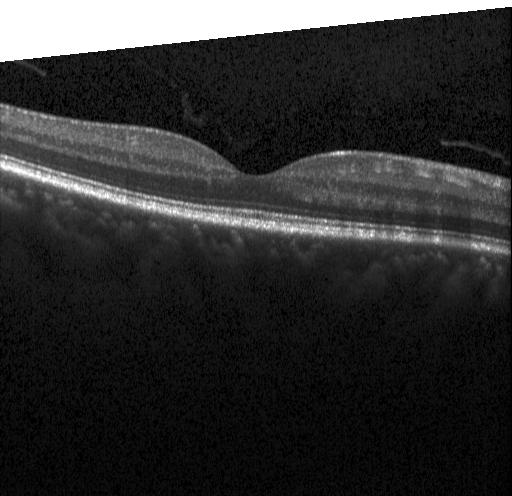 SD-OCT; optical coherence tomography scan
Impression: no CNV, DME, or drusen.